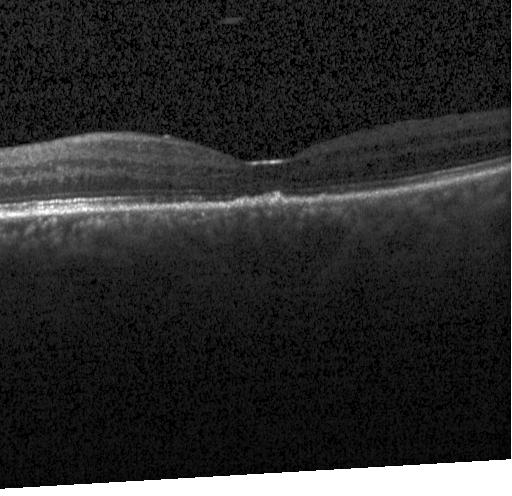

Retinal OCT cross-section. Drusen.